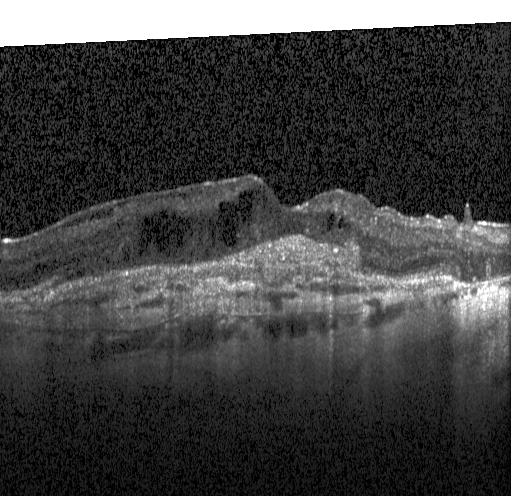 Impression: CNV.